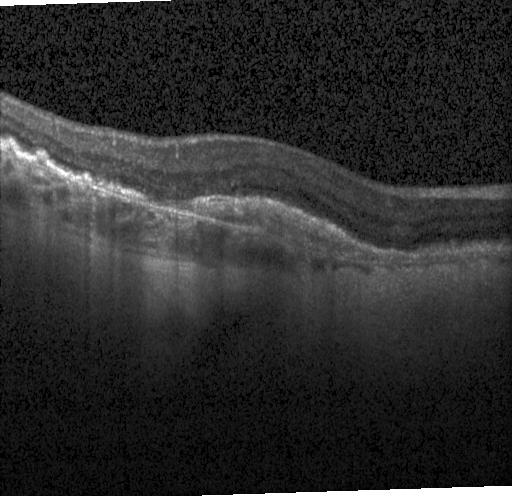
Acquired on a Heidelberg Spectralis. Retinal OCT B-scan.
Dx: CNV.